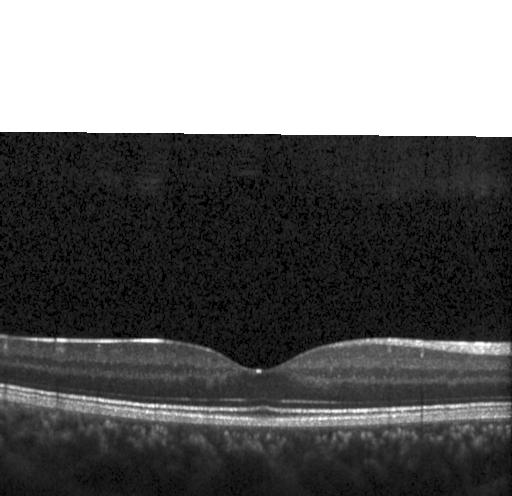
Horizontal scan through the fovea, retinal OCT cross-section — Finding: no choroidal neovascularization, no diabetic macular edema, and no drusen.